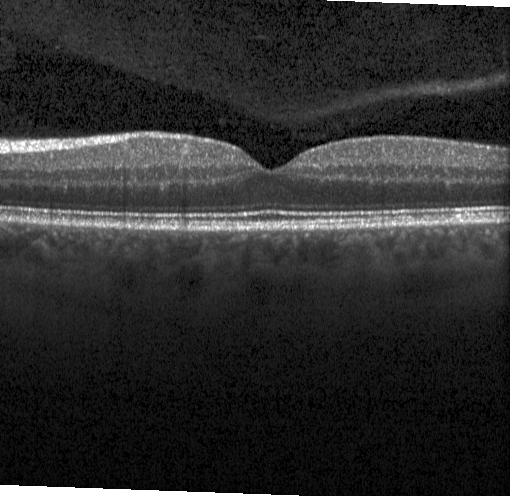 Horizontal scan through the fovea, spectral-domain optical coherence tomography, Heidelberg Spectralis OCT system, retinal OCT B-scan — Impression: neither choroidal neovascularization, diabetic macular edema, nor drusen.